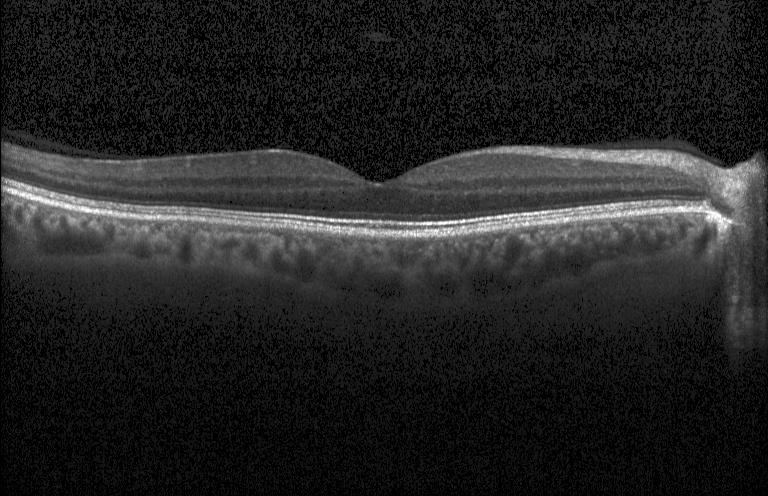

Retinal OCT cross-section. Macular OCT: no choroidal neovascularization, diabetic macular edema, or drusen.